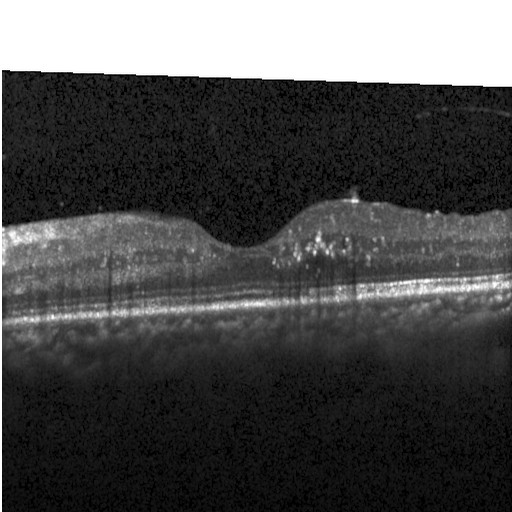
Spectral-domain optical coherence tomography; Heidelberg Spectralis OCT system; horizontal scan through the fovea; OCT line scan. Dx: diabetic macular edema (DME).